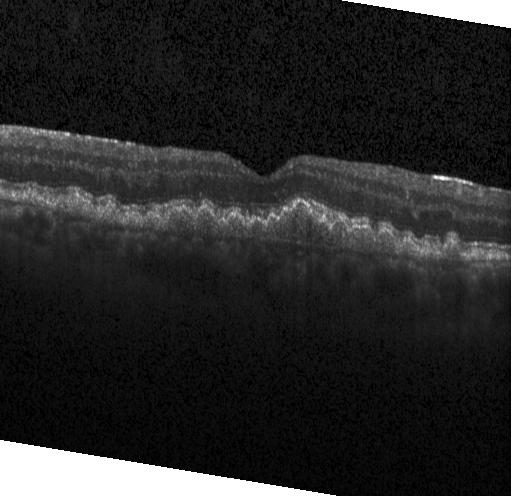 Retinal OCT B-scan — This B-scan demonstrates a choroidal neovascular membrane.